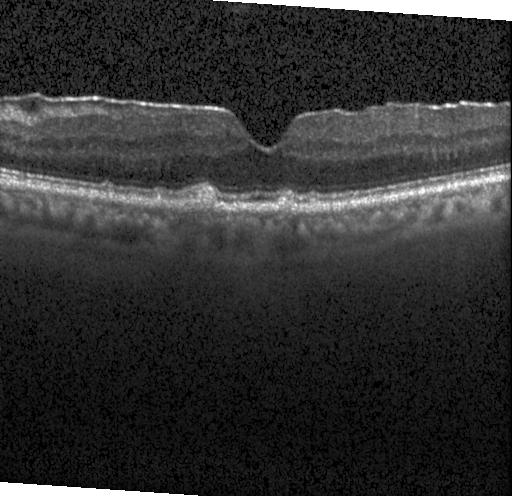
Retinal OCT B-scan; Heidelberg Spectralis OCT system
Macular OCT: drusen.